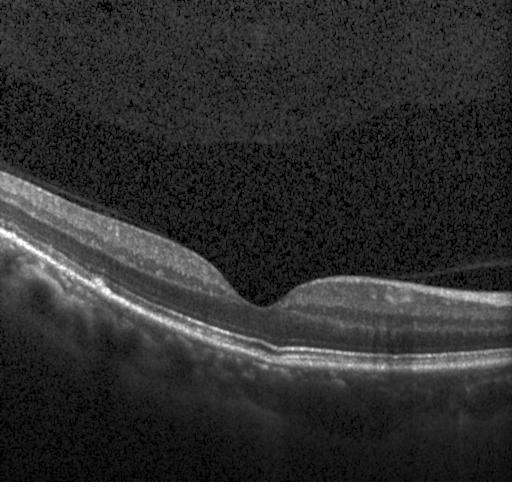

Finding: sub-RPE drusenoid deposits.